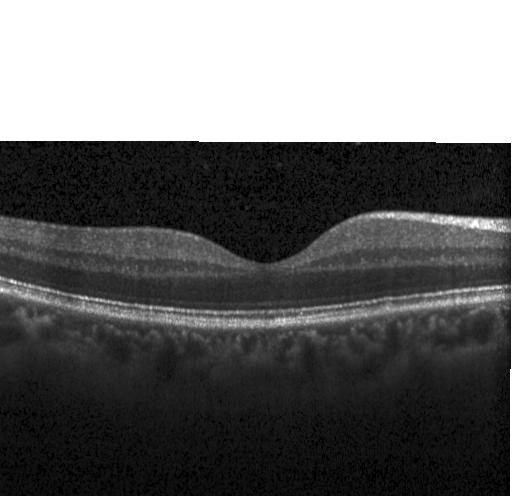 Optical coherence tomography scan.
OCT finding: neither choroidal neovascularization, diabetic macular edema, nor drusen.